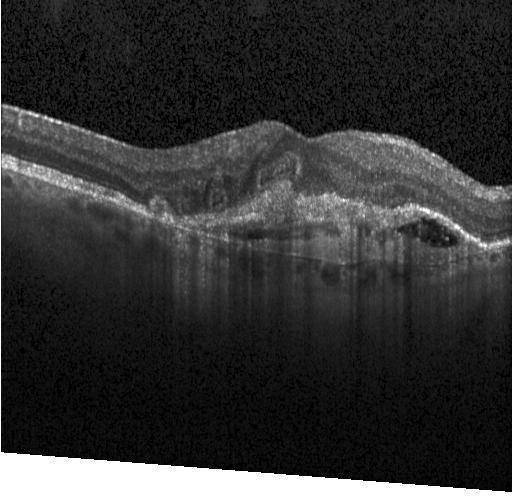

Macular scan, spectral-domain OCT, Heidelberg Spectralis, retinal OCT B-scan — Macular OCT: a choroidal neovascular membrane.